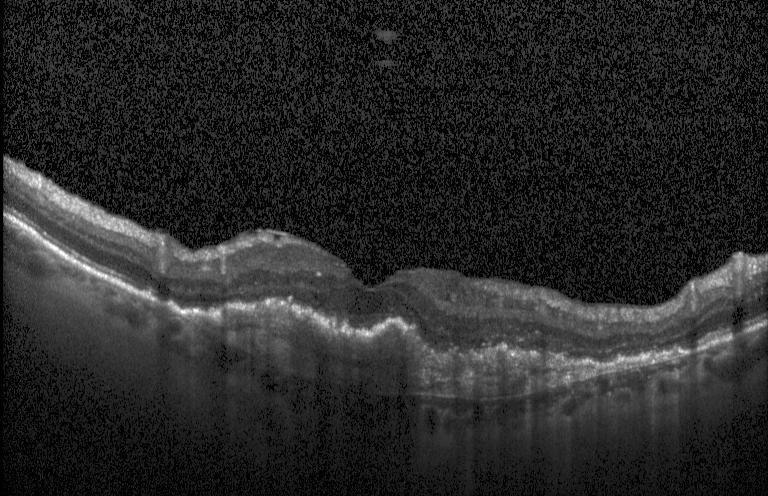 Diagnosis: choroidal neovascularization (CNV).